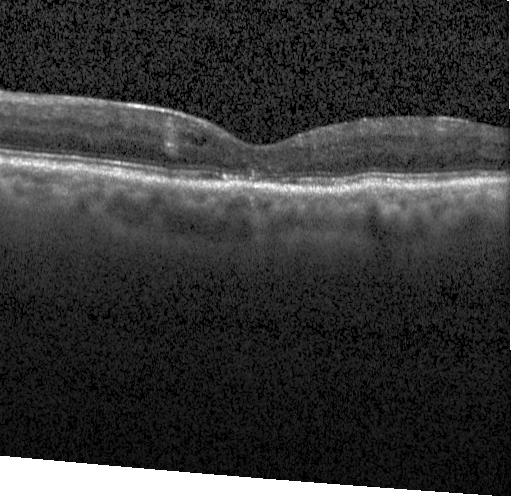 OCT B-scan, macular scan, Heidelberg Spectralis, spectral-domain OCT.
Diagnosis: diabetic macular edema.